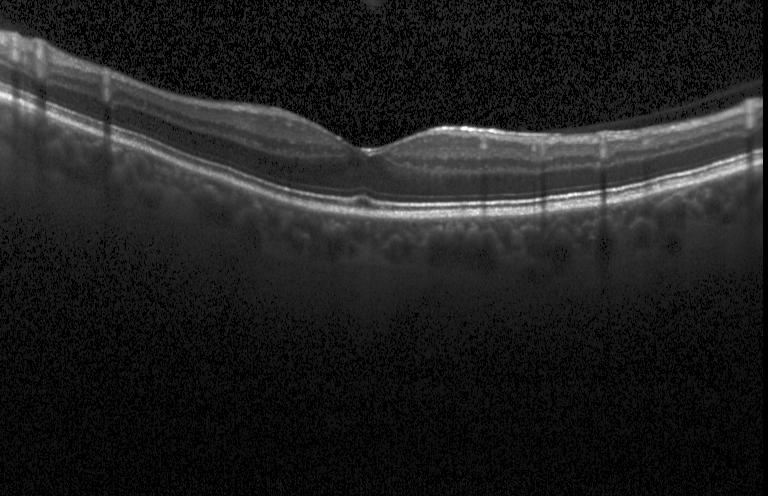
Spectral-domain OCT B-scan: no choroidal neovascularization, no diabetic macular edema, and no drusen.